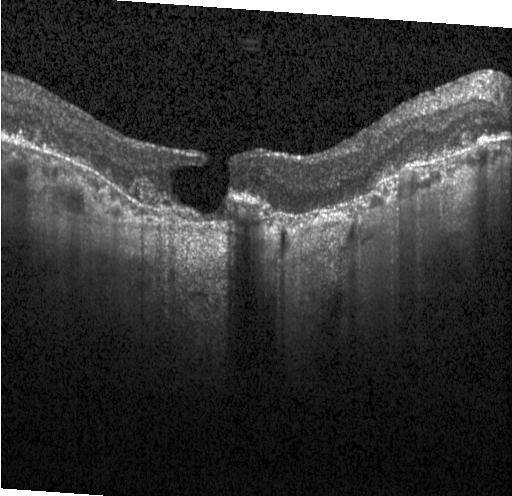

Retinal OCT B-scan.
The scan shows choroidal neovascularization (CNV).